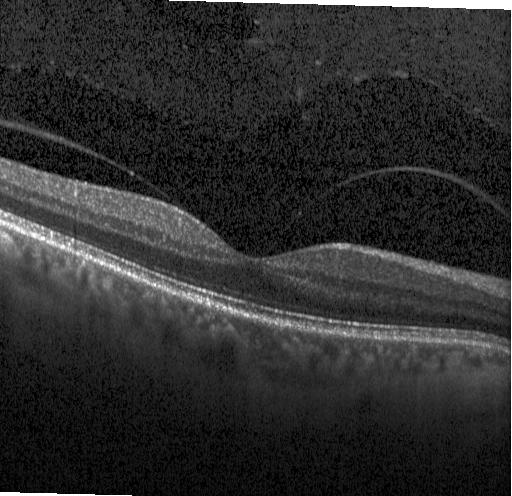

Spectral-domain optical coherence tomography · Heidelberg Spectralis · OCT B-scan. Finding: no choroidal neovascularization, no diabetic macular edema, and no drusen.